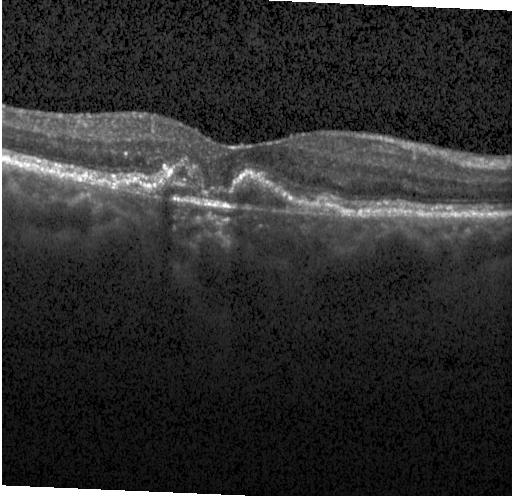 Heidelberg Spectralis; spectral-domain optical coherence tomography; OCT B-scan; through the macula
Assessment: a choroidal neovascular membrane.